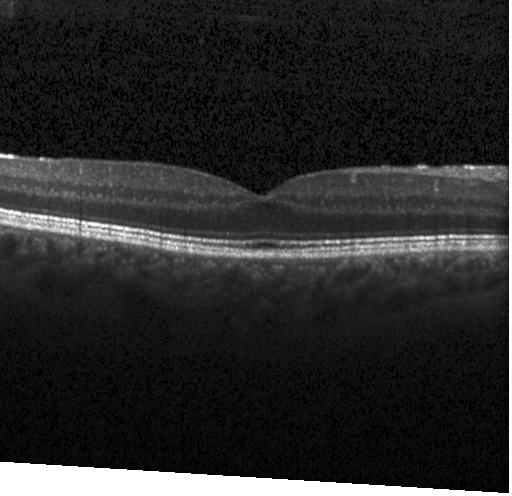
Macular OCT: no evidence of CNV, DME, or drusen.